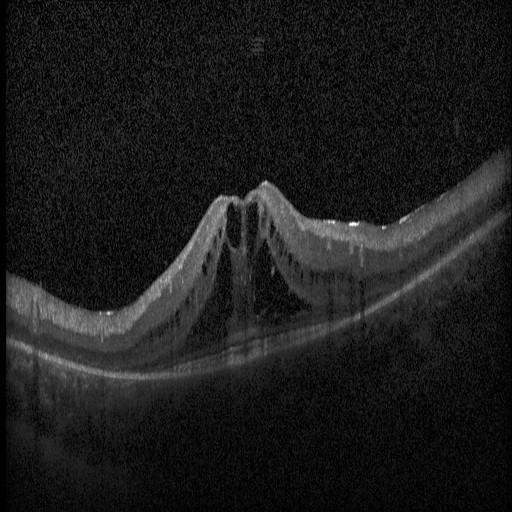
Retinal OCT cross-section, through the macula — Impression: diabetic macular edema (DME).